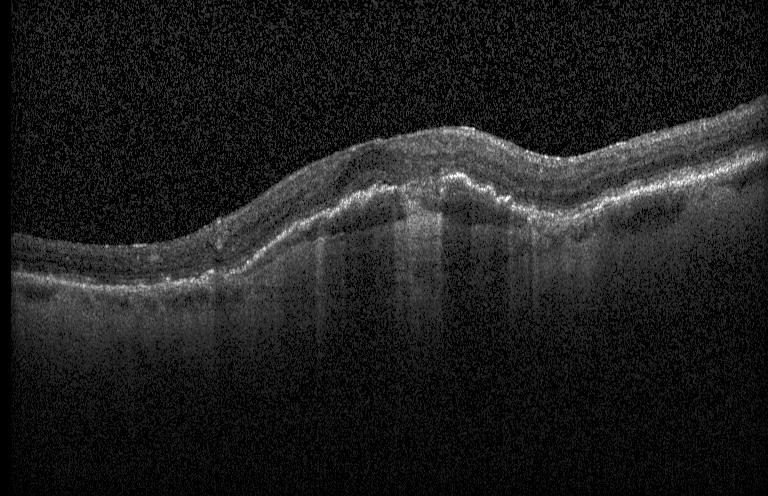
OCT finding: choroidal neovascularization (CNV).